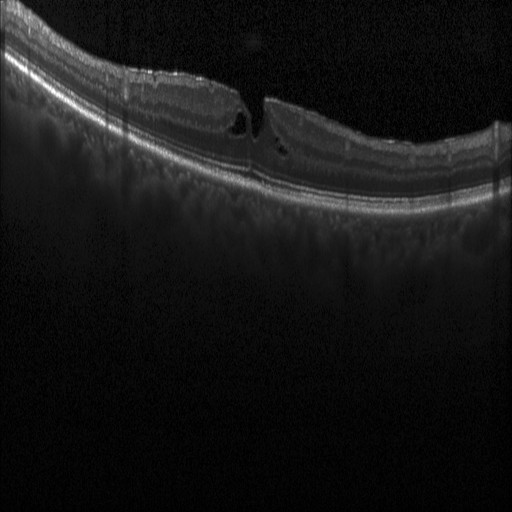
Horizontal scan through the fovea · spectral-domain OCT · retinal OCT cross-section
Assessment: diabetic macular edema.